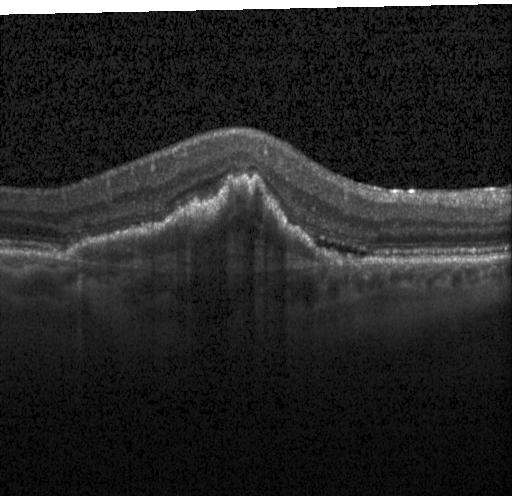
Spectral-domain optical coherence tomography. OCT B-scan. Centered on the fovea — OCT finding: a choroidal neovascular membrane.